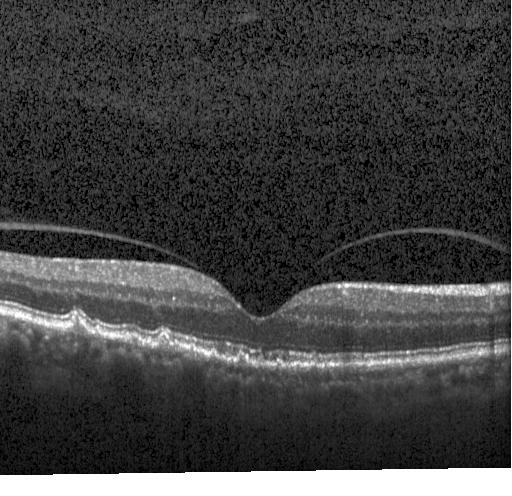 Diagnosis: multiple drusen.